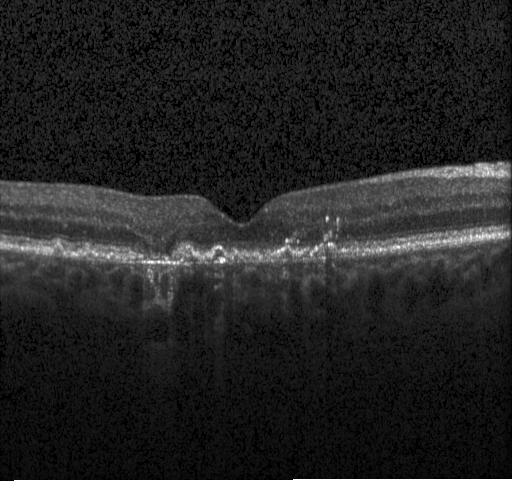

Heidelberg Spectralis; spectral-domain optical coherence tomography; optical coherence tomography B-scan
The scan shows CNV.